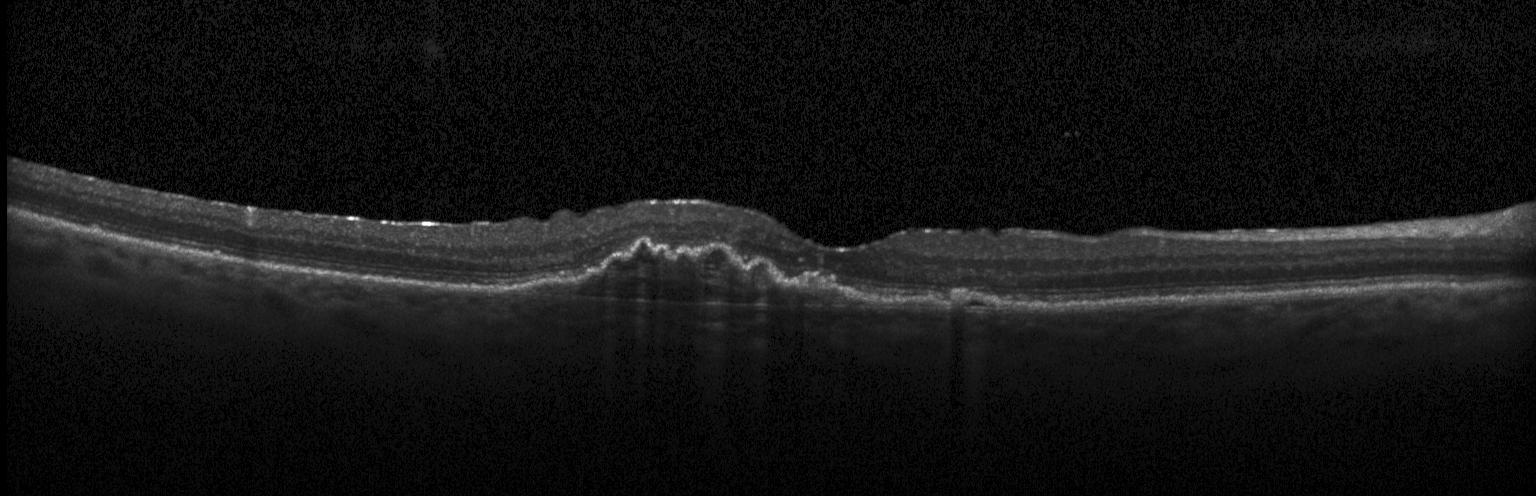

Impression: a choroidal neovascular membrane.